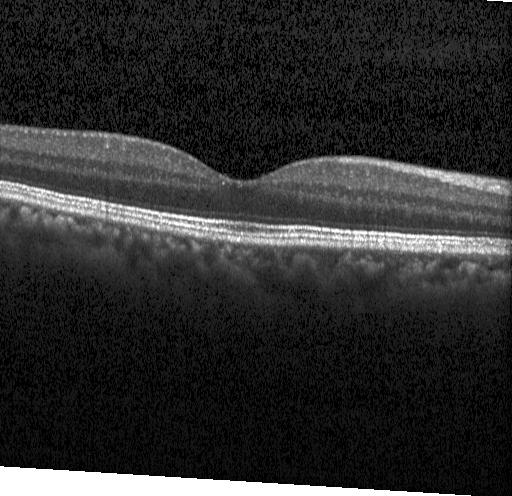

Diagnosis: no CNV, no DME, and no drusen.